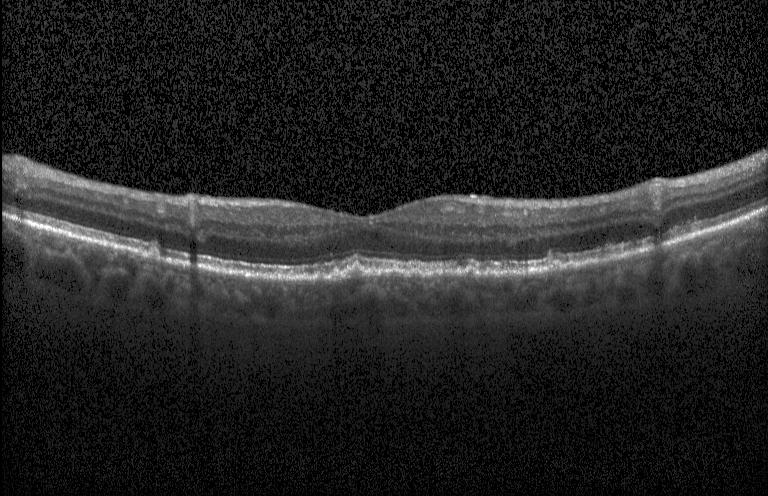
Impression: drusen.